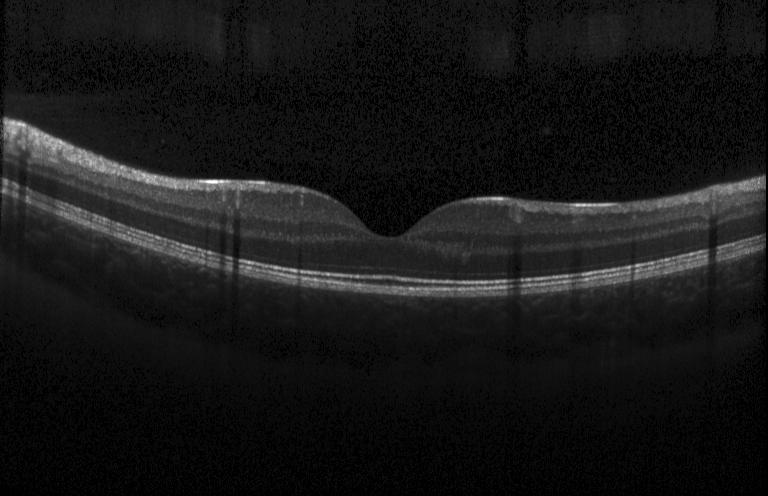 Centered on the fovea. Heidelberg Spectralis. Spectral-domain OCT. Optical coherence tomography scan. Assessment: no CNV, no DME, and no drusen.